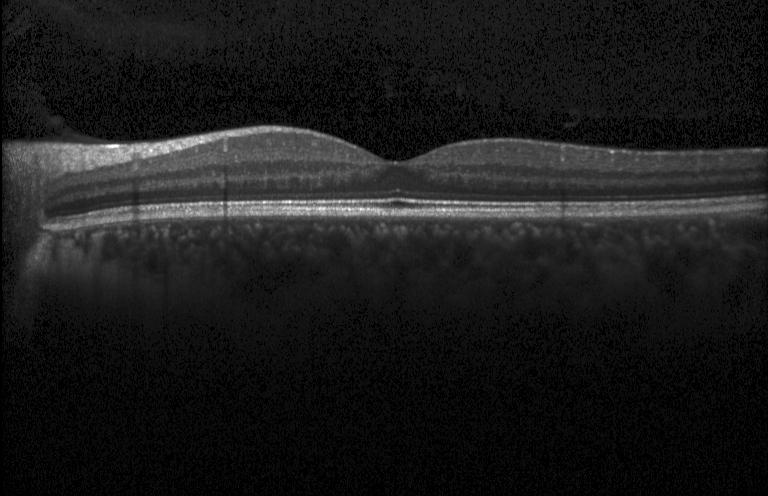 Optical coherence tomography scan. OCT finding: no CNV, no DME, and no drusen.